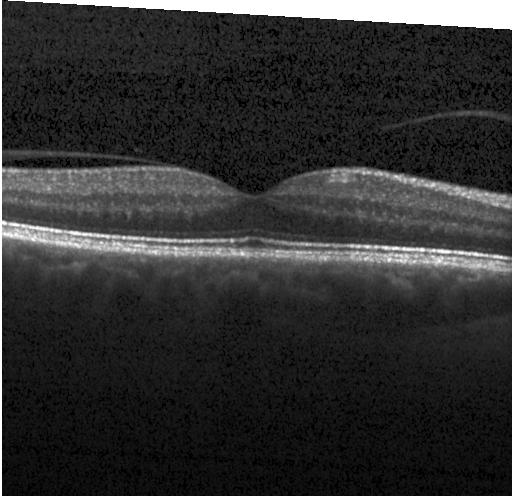 Macular OCT: no choroidal neovascularization, no diabetic macular edema, and no drusen.